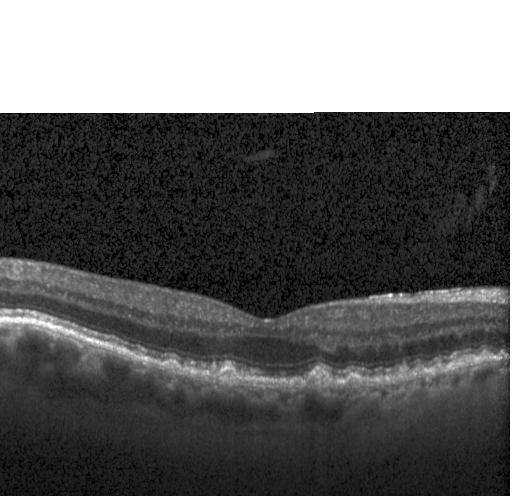

OCT B-scan showing multiple drusen.